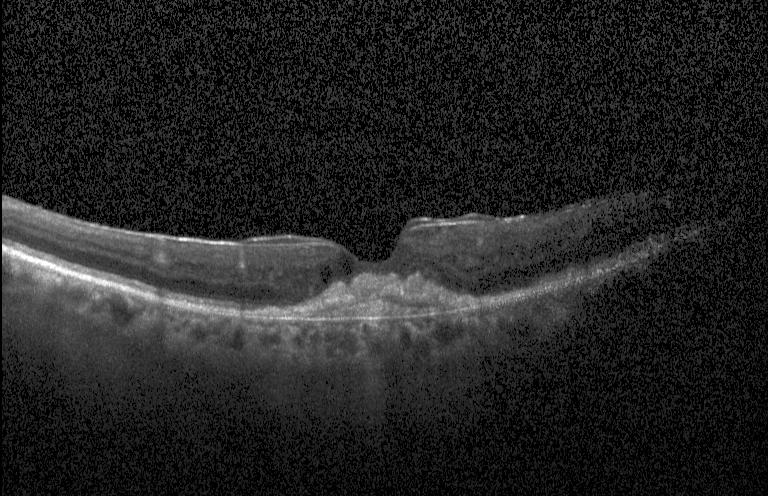

Spectral-domain optical coherence tomography · through the macula · Heidelberg Spectralis · optical coherence tomography B-scan — Diagnosis: choroidal neovascularization.